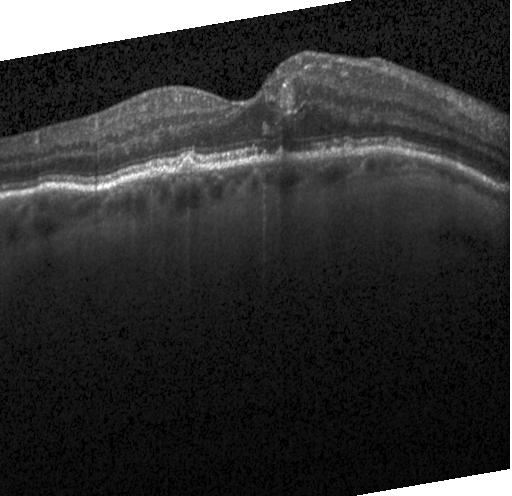 Retinal OCT cross-section showing drusen.